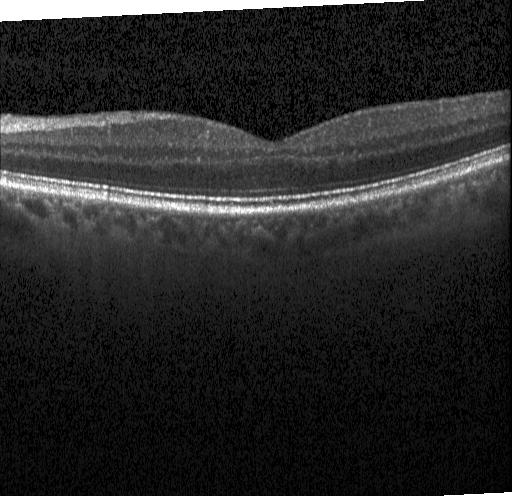 OCT line scan — OCT finding: no CNV, DME, or drusen.